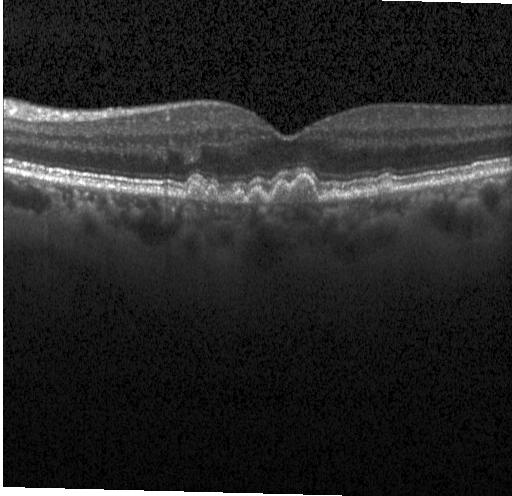
Multiple drusen.